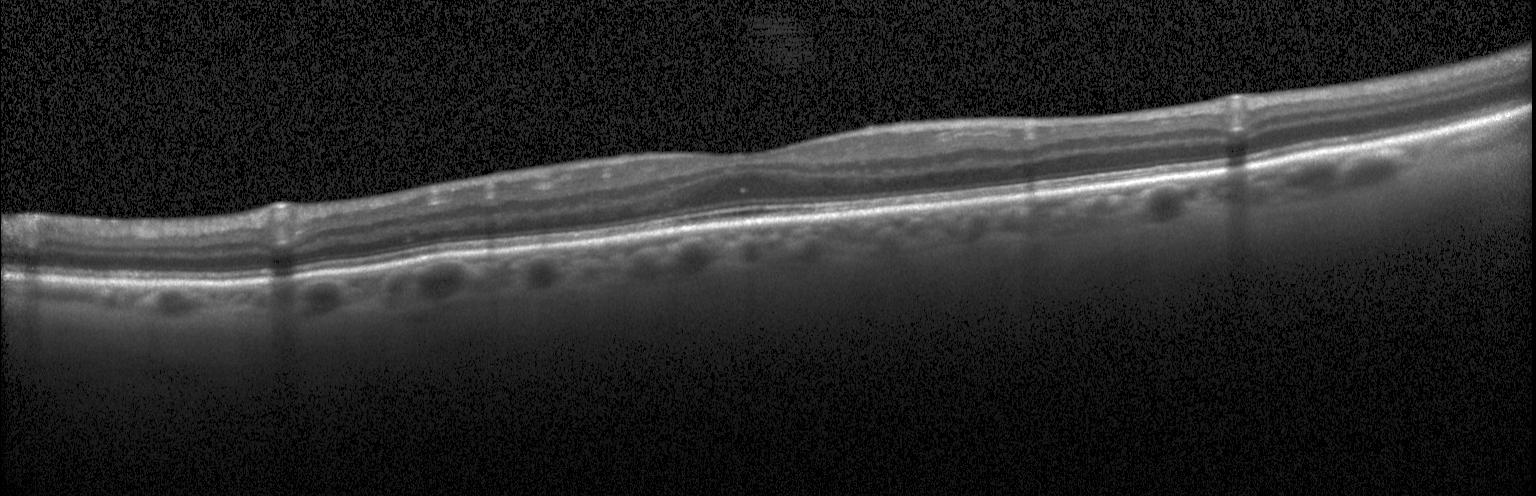

Spectral-domain OCT B-scan: no choroidal neovascularization, diabetic macular edema, or drusen.